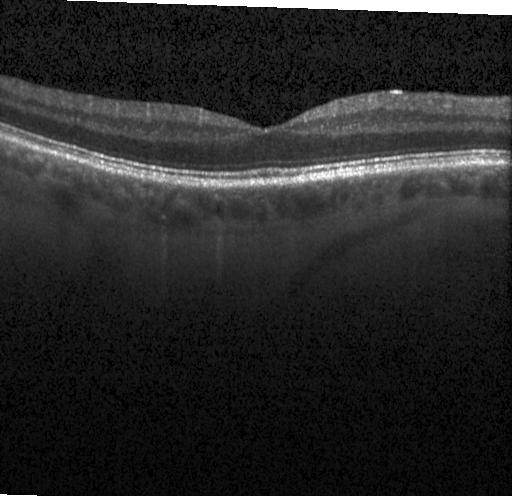
Heidelberg Spectralis, retinal OCT B-scan
Dx: no evidence of choroidal neovascularization, diabetic macular edema, or drusen.